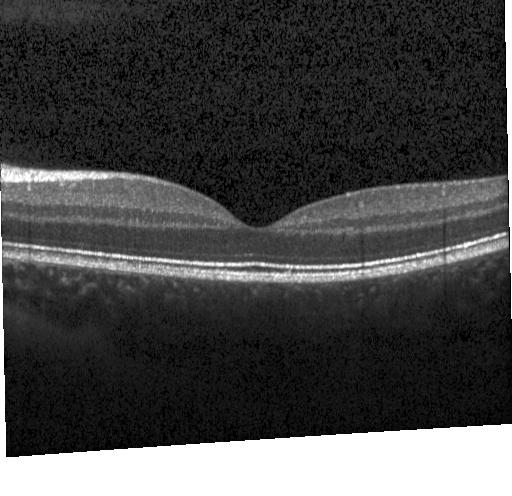 Through the macula · Heidelberg Spectralis · retinal OCT cross-section · SD-OCT
This B-scan demonstrates neither choroidal neovascularization, diabetic macular edema, nor drusen.